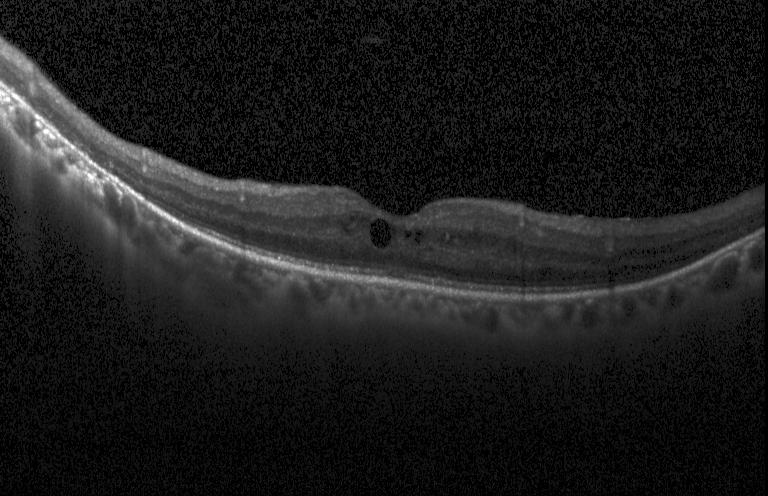

Acquired on a Heidelberg Spectralis · optical coherence tomography scan · fovea-centered.
Dx: diabetic macular edema (DME).